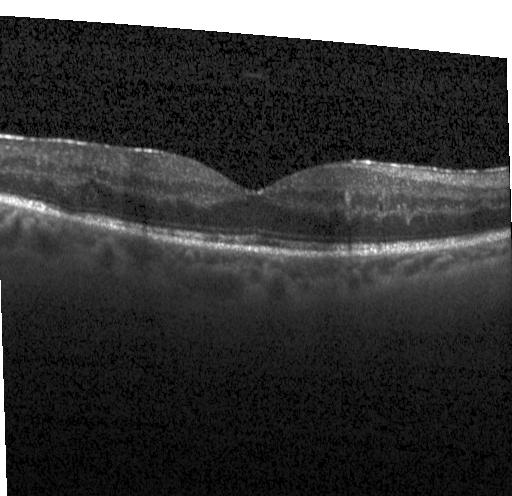

Impression: no evidence of CNV, DME, or drusen.